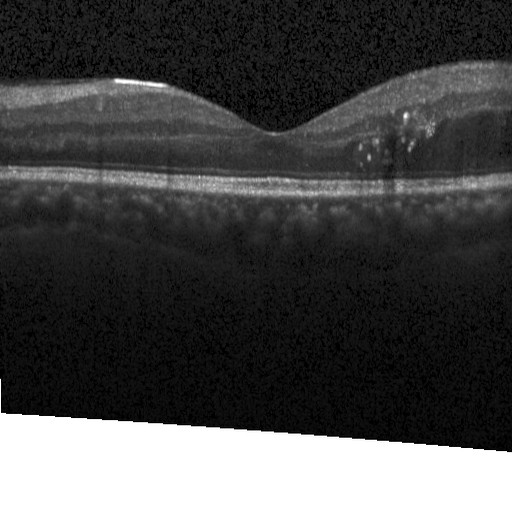
Impression: diabetic macular edema (DME).